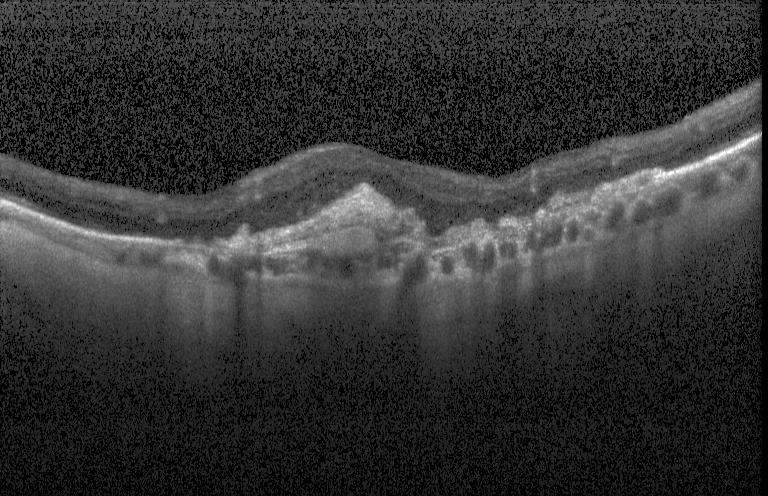
OCT B-scan showing CNV.